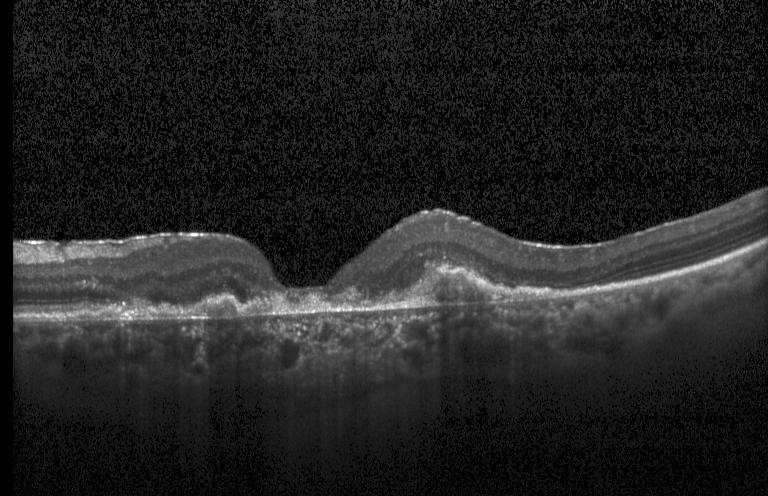 CNV.